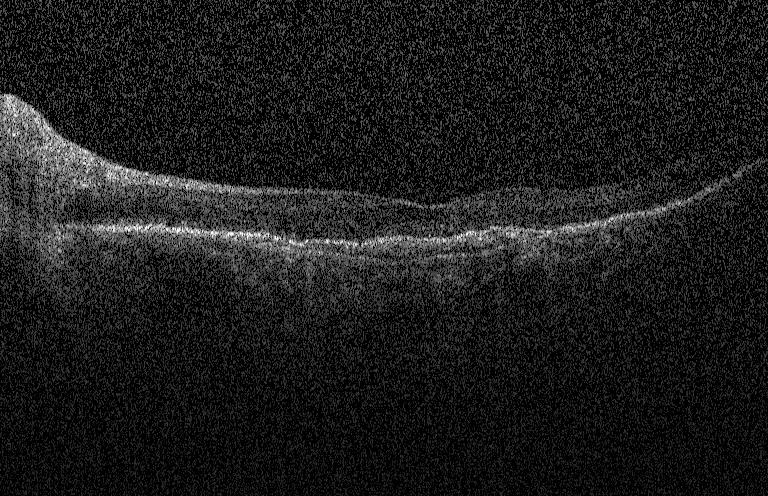
Centered on the fovea · retinal OCT B-scan · spectral-domain optical coherence tomography
Finding: a choroidal neovascular membrane.